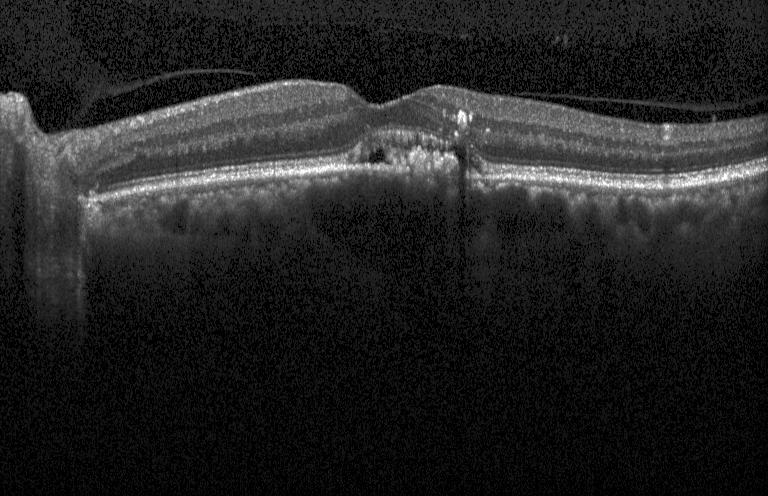
OCT line scan. Heidelberg Spectralis OCT system. SD-OCT — OCT finding: a choroidal neovascular membrane.